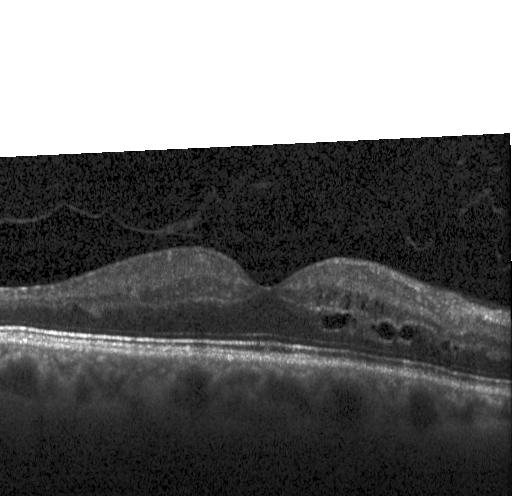 Acquired on a Heidelberg Spectralis; OCT line scan; spectral-domain optical coherence tomography; macular scan. Macular OCT: diabetic macular edema (DME).